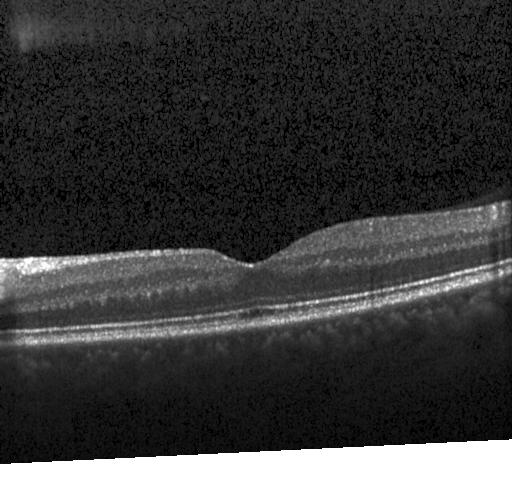

Fovea-centered · optical coherence tomography B-scan. The scan shows no evidence of choroidal neovascularization, diabetic macular edema, or drusen.